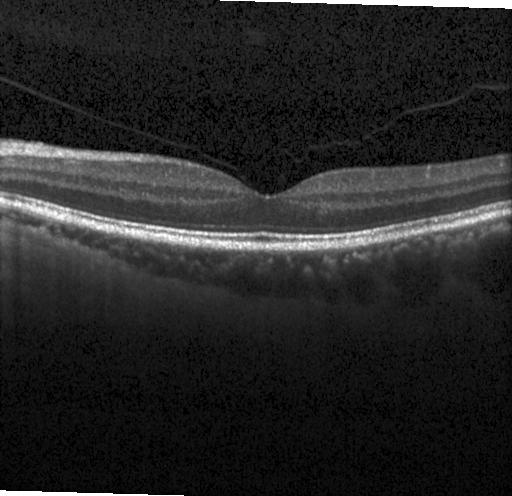
Retinal OCT cross-section; fovea-centered. OCT finding: no evidence of choroidal neovascularization, diabetic macular edema, or drusen.